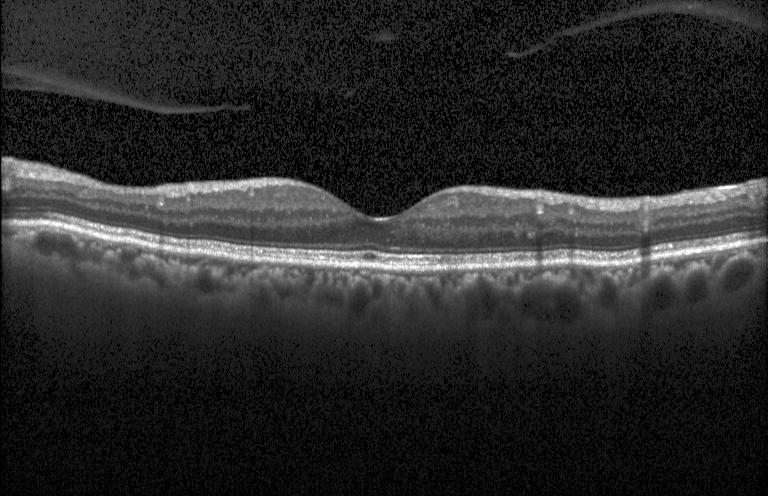 Neither CNV, DME, nor drusen.